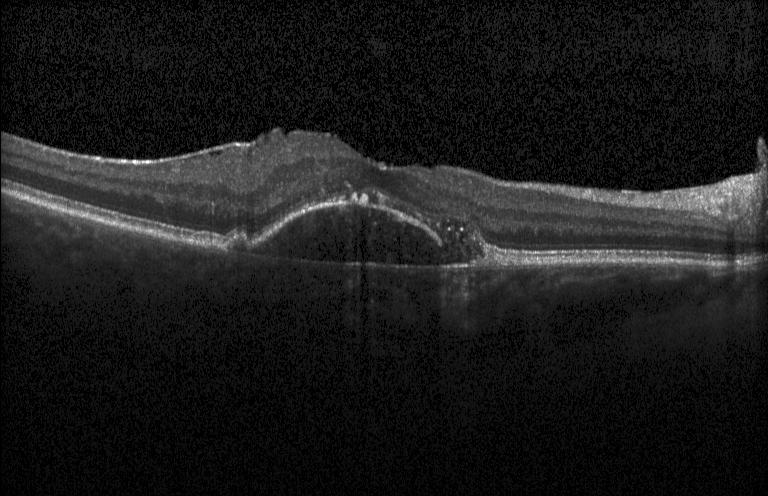 Retinal OCT B-scan.
Diagnosis: a choroidal neovascular membrane.